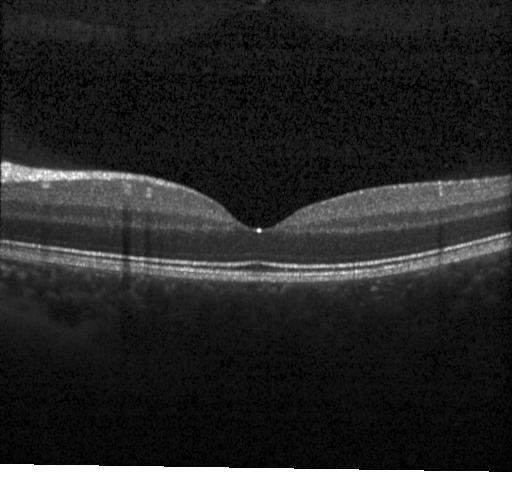
OCT finding: neither CNV, DME, nor drusen.